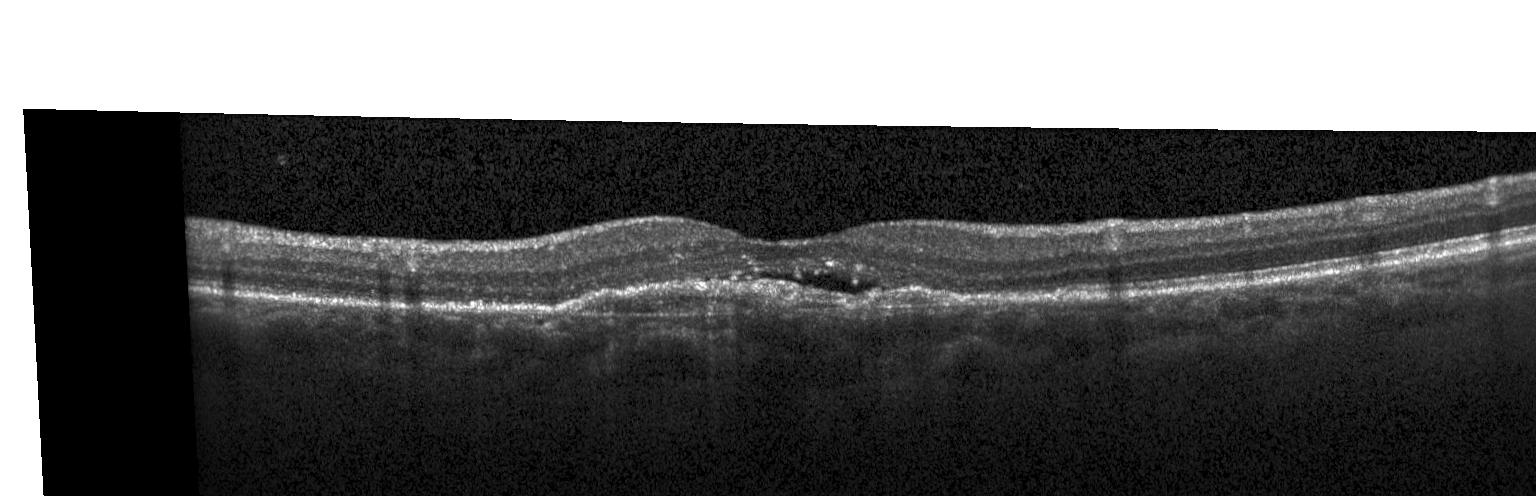 Heidelberg Spectralis OCT system, OCT line scan, spectral-domain optical coherence tomography. The scan shows choroidal neovascularization (CNV).